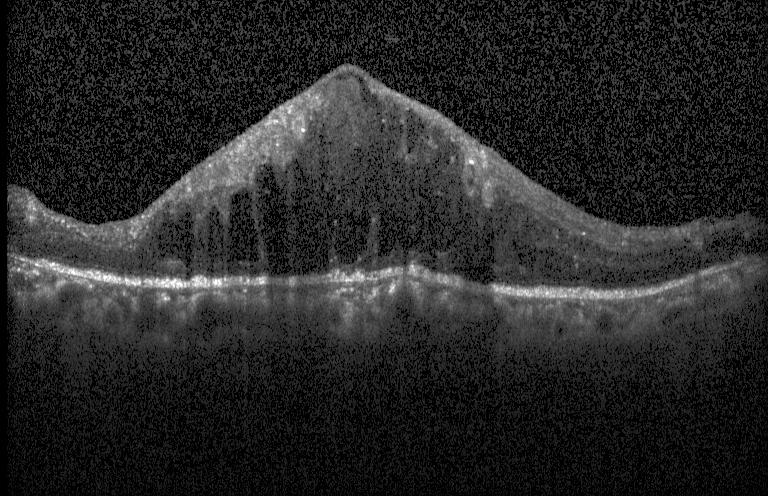 Fovea-centered · spectral-domain OCT · OCT B-scan
Dx: DME.